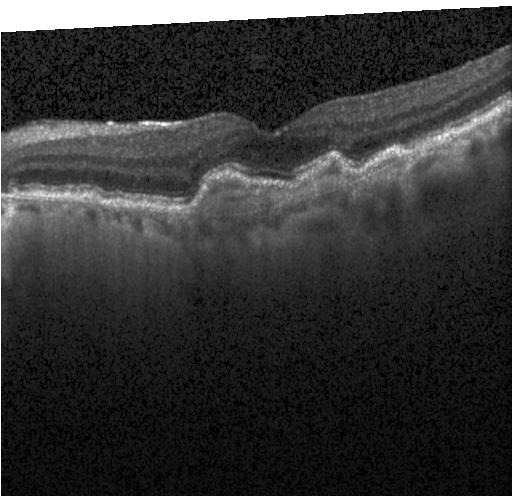
Retinal OCT B-scan. Instrument: Heidelberg Spectralis.
Macular OCT: choroidal neovascularization.